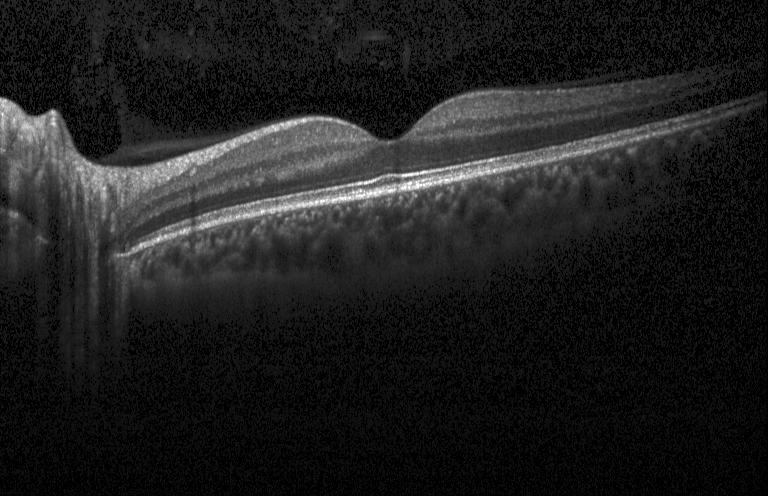 This B-scan demonstrates no choroidal neovascularization, diabetic macular edema, or drusen.